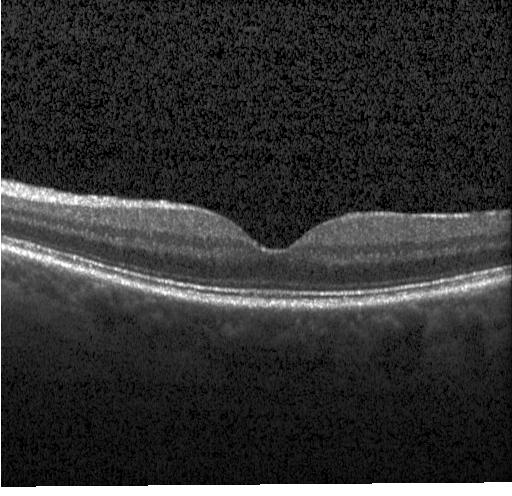

OCT line scan. Assessment: no evidence of choroidal neovascularization, diabetic macular edema, or drusen.